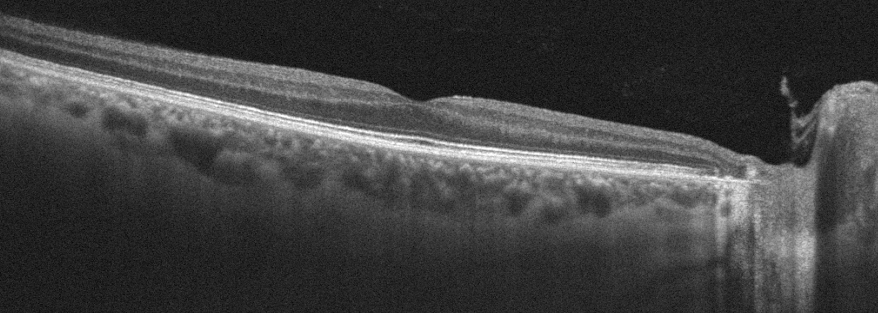
Retinal OCT B-scan · fovea-centered.
The scan shows no evidence of AMD, DME, ERM, RAO, RVO, or VID.